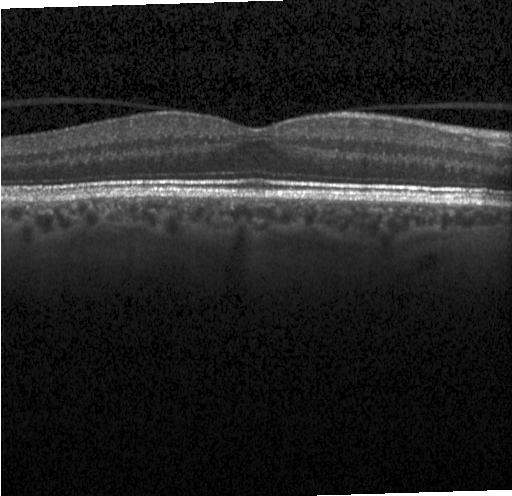

Optical coherence tomography B-scan.
OCT finding: neither choroidal neovascularization, diabetic macular edema, nor drusen.